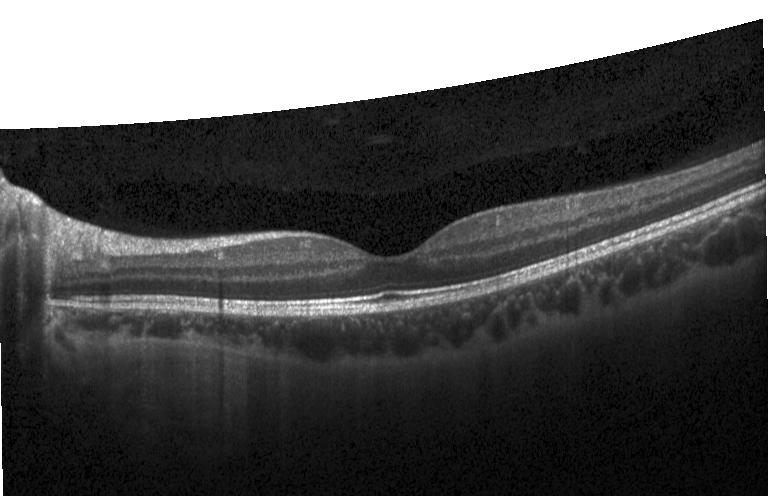

OCT scan showing no evidence of choroidal neovascularization, diabetic macular edema, or drusen.